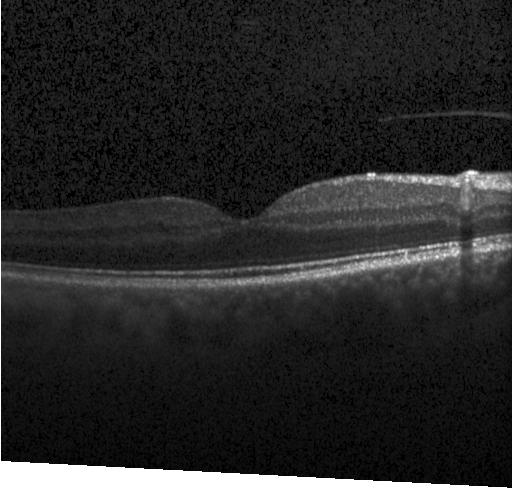
Retinal OCT B-scan
Diagnosis: no choroidal neovascularization, no diabetic macular edema, and no drusen.